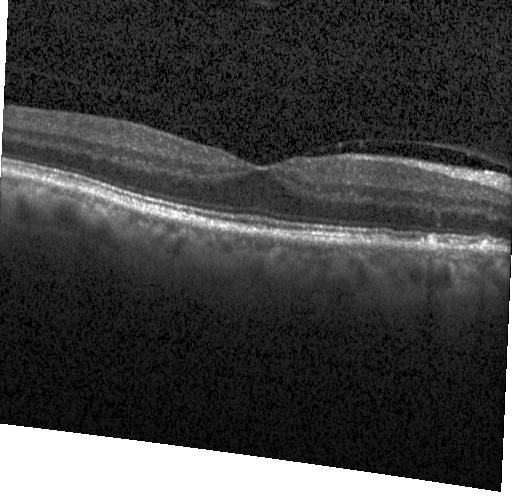
OCT line scan · through the macula. Impression: multiple drusen.